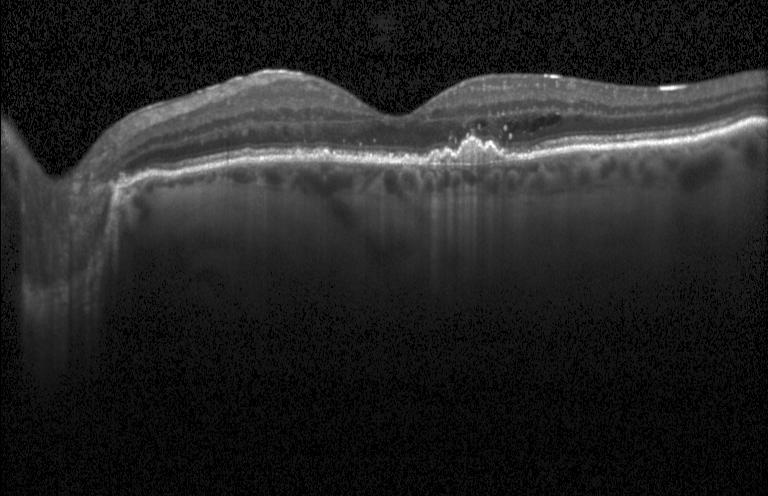

OCT finding: sub-RPE drusenoid deposits.